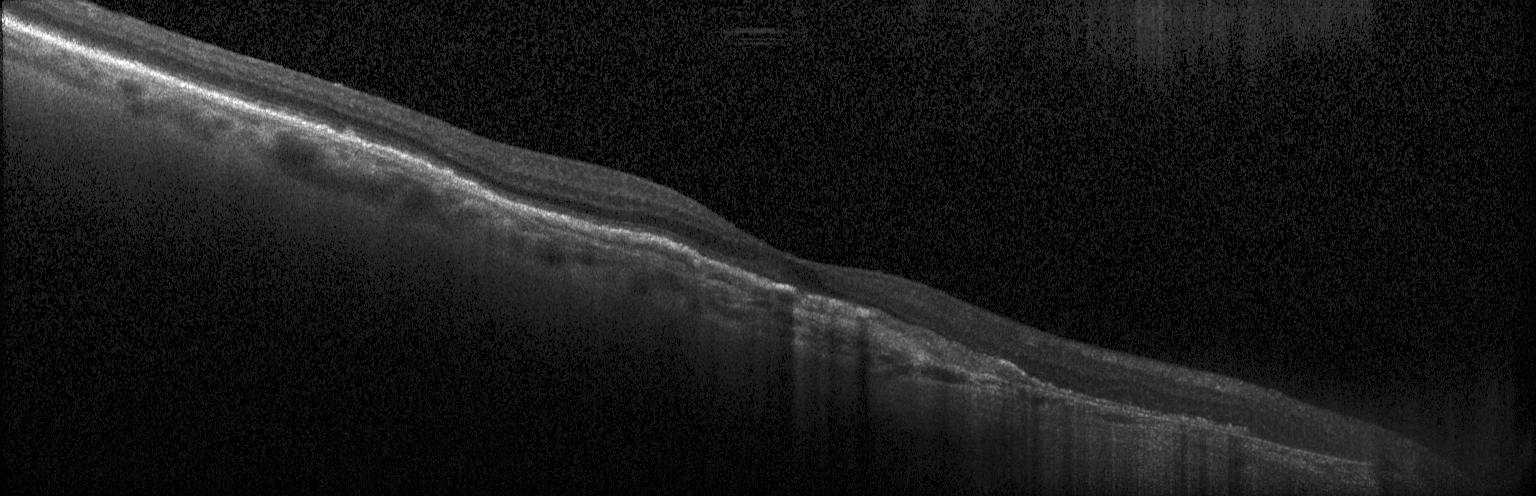
Optical coherence tomography B-scan
Diagnosis: a choroidal neovascular membrane.